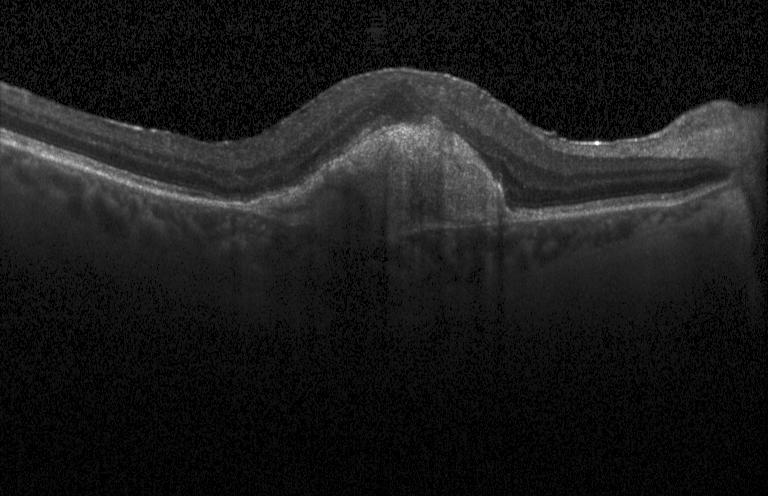 Retinal OCT B-scan. Diagnosis: a choroidal neovascular membrane.